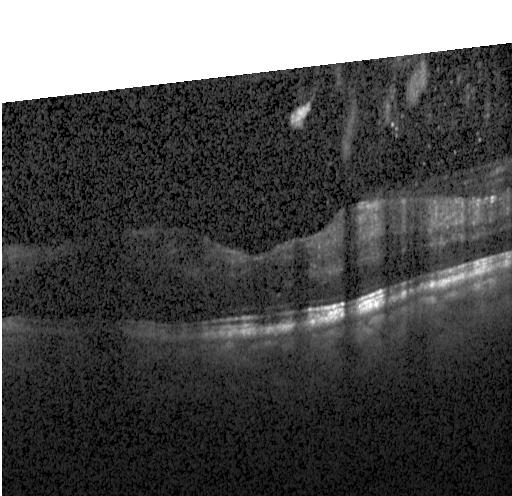 Retinal OCT cross-section.
Neither choroidal neovascularization, diabetic macular edema, nor drusen.